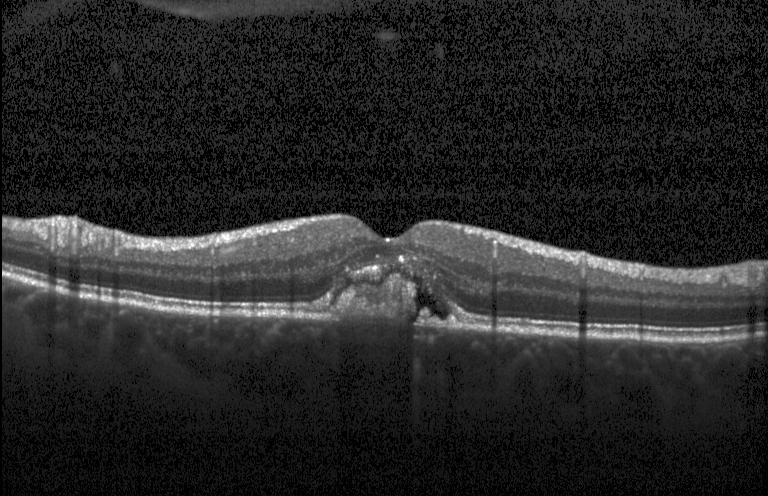 OCT finding: choroidal neovascularization.